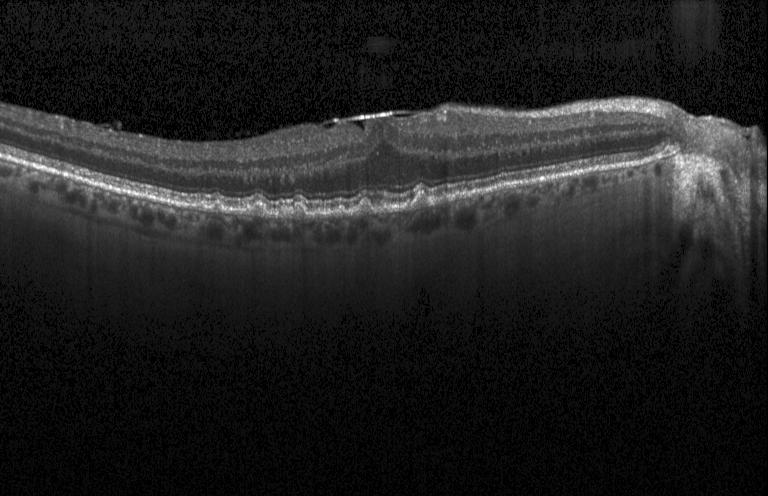 Macular OCT demonstrating drusen.